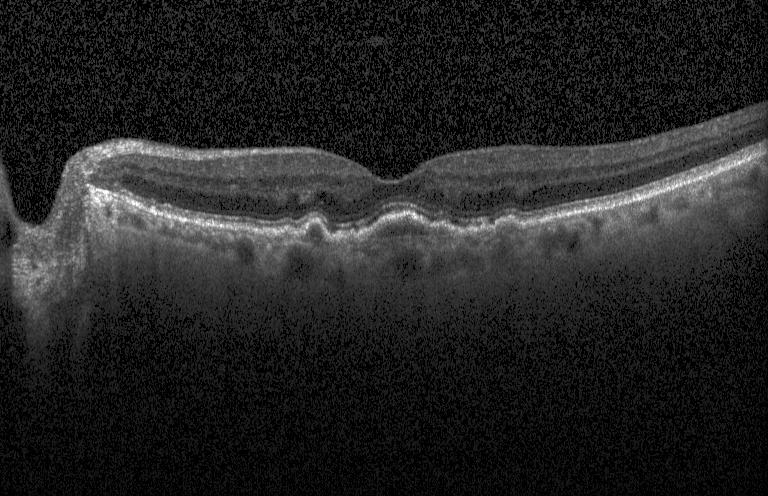 Heidelberg Spectralis OCT system · macular scan · retinal OCT cross-section · SD-OCT.
A choroidal neovascular membrane.